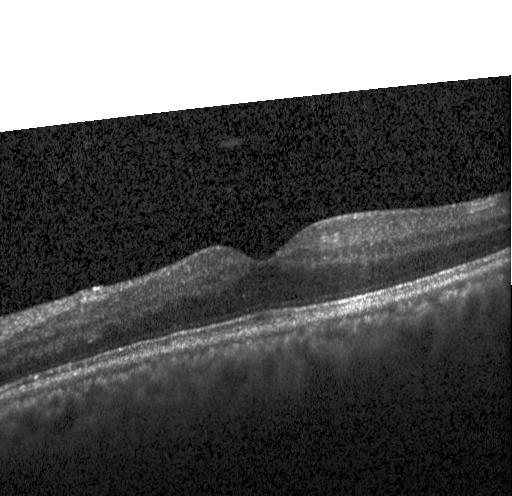

Macular OCT demonstrating no choroidal neovascularization, diabetic macular edema, or drusen.